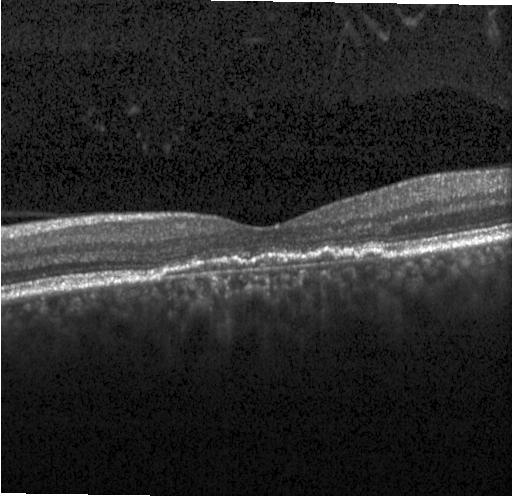
Finding: CNV.